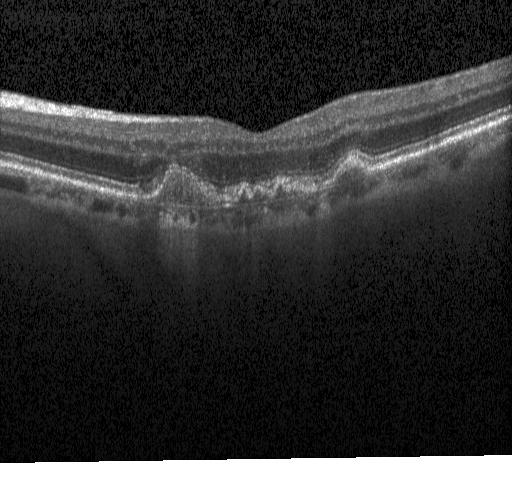

Optical coherence tomography scan, macular scan.
This B-scan demonstrates a choroidal neovascular membrane.